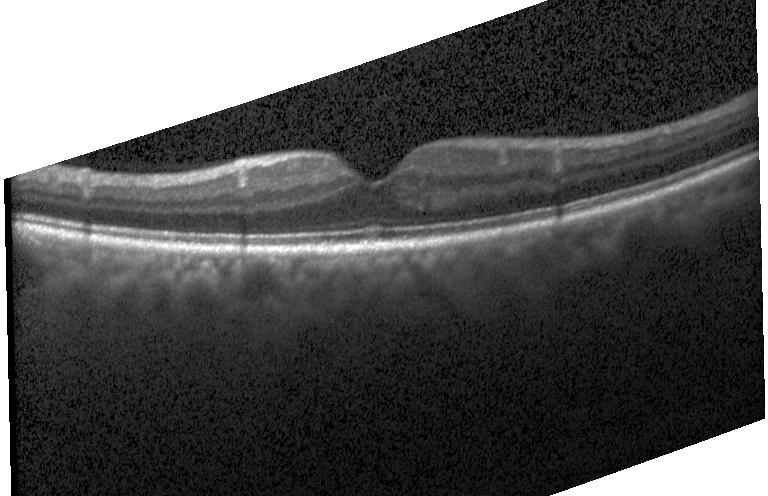
Retinal OCT B-scan, spectral-domain OCT
No choroidal neovascularization, diabetic macular edema, or drusen.